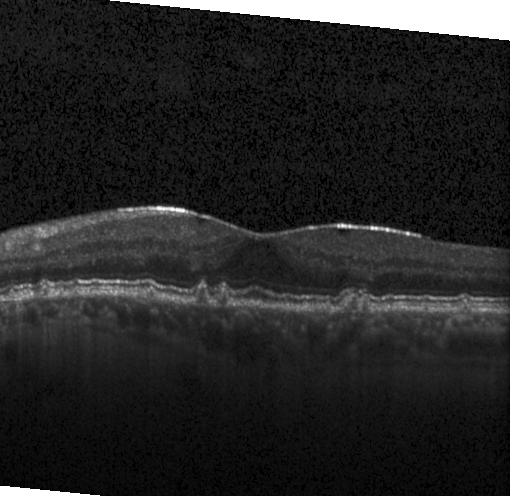

Macular scan, optical coherence tomography scan
This B-scan demonstrates sub-RPE drusenoid deposits.